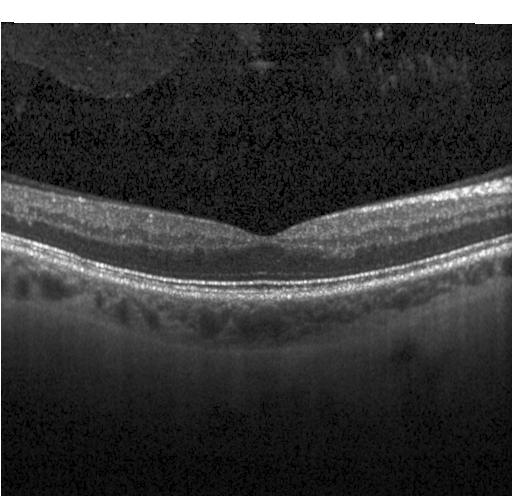 Dx: no CNV, no DME, and no drusen.